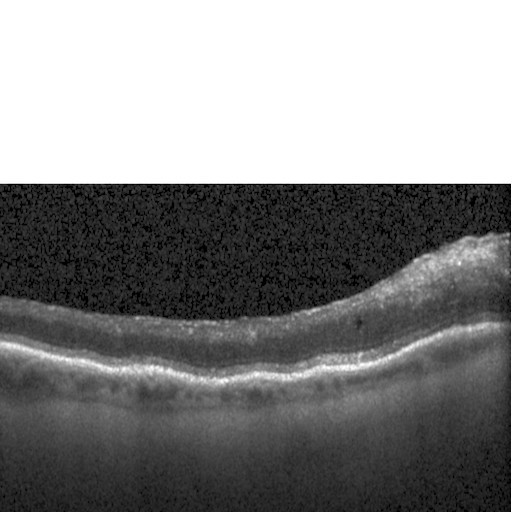
Optical coherence tomography scan, fovea-centered.
Diabetic macular edema.